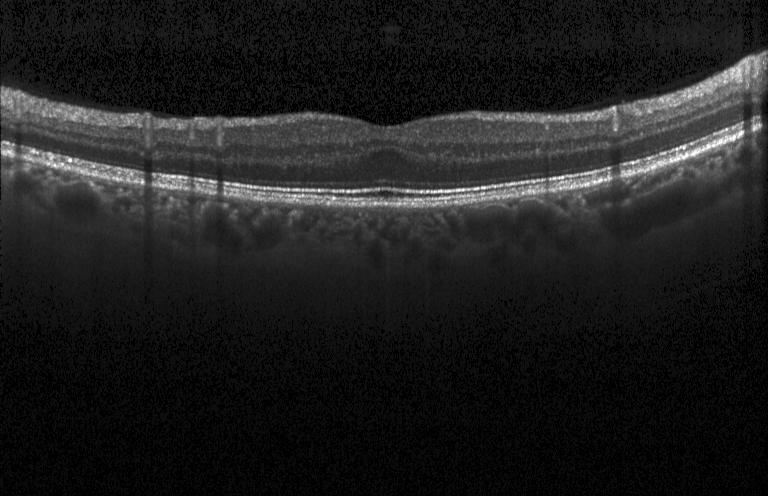 Macular OCT demonstrating no CNV, DME, or drusen.